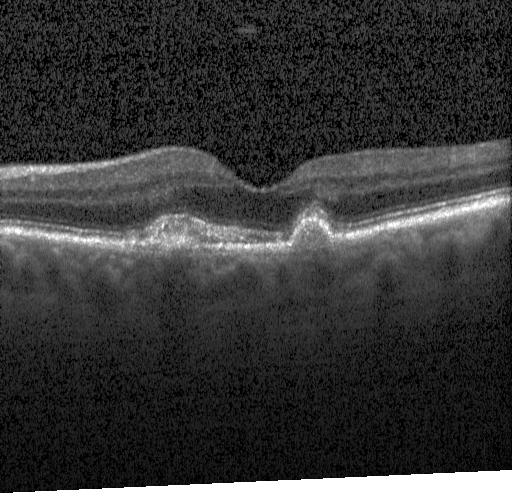 OCT scan showing a choroidal neovascular membrane.